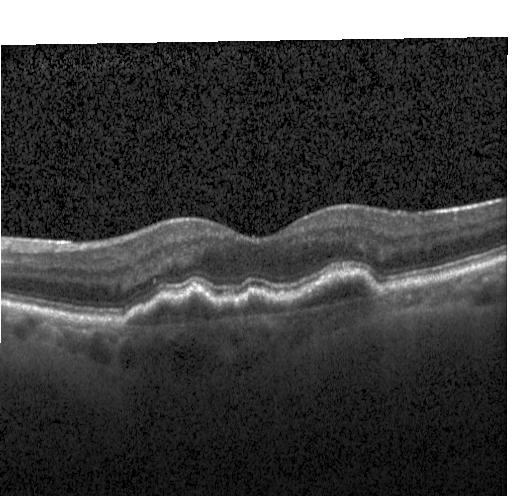
Instrument: Heidelberg Spectralis. Macular scan. Spectral-domain optical coherence tomography. OCT line scan.
Assessment: a choroidal neovascular membrane.